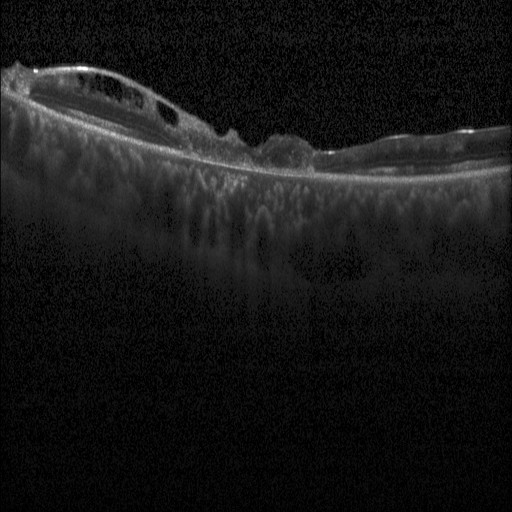

Heidelberg Spectralis; SD-OCT; OCT line scan; fovea-centered — This B-scan demonstrates DME.